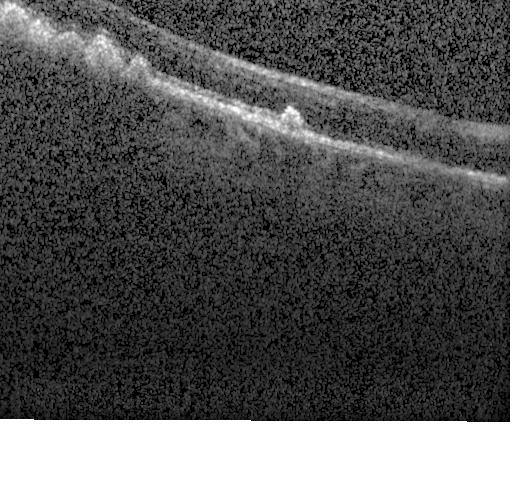

Heidelberg Spectralis OCT system; retinal OCT cross-section.
Finding: drusen.